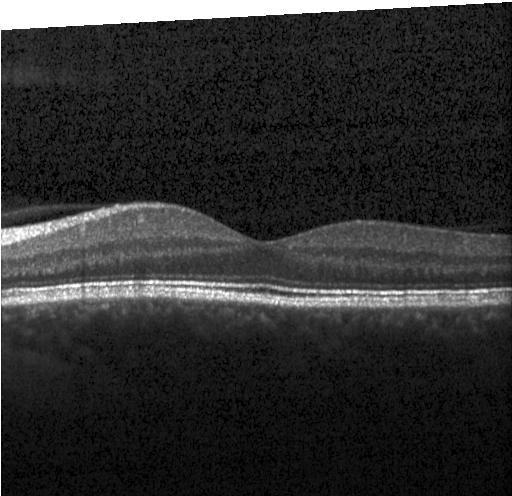 Spectral-domain OCT. Centered on the fovea. Optical coherence tomography B-scan.
Diagnosis: no CNV, no DME, and no drusen.